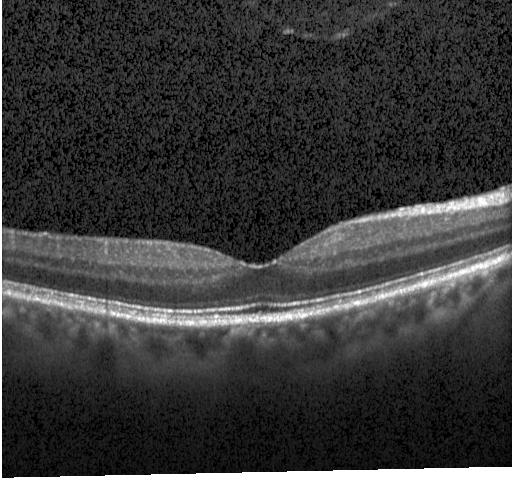

Retinal OCT B-scan, spectral-domain OCT, acquired on a Heidelberg Spectralis.
Finding: no choroidal neovascularization, diabetic macular edema, or drusen.